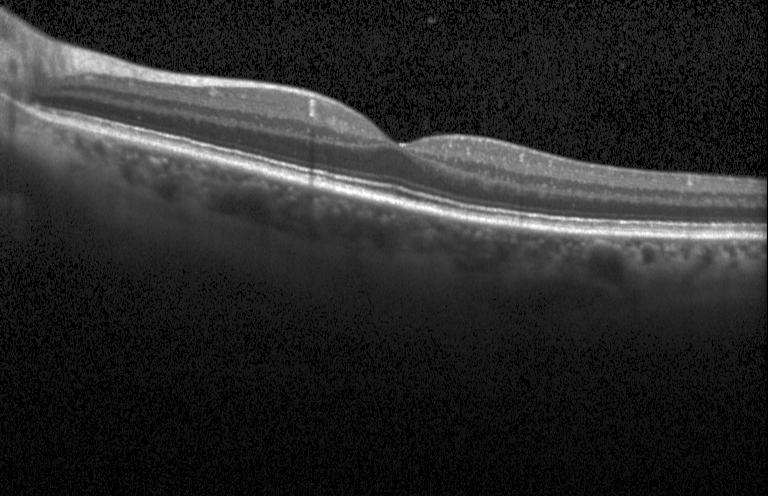 Dx: no choroidal neovascularization, no diabetic macular edema, and no drusen.